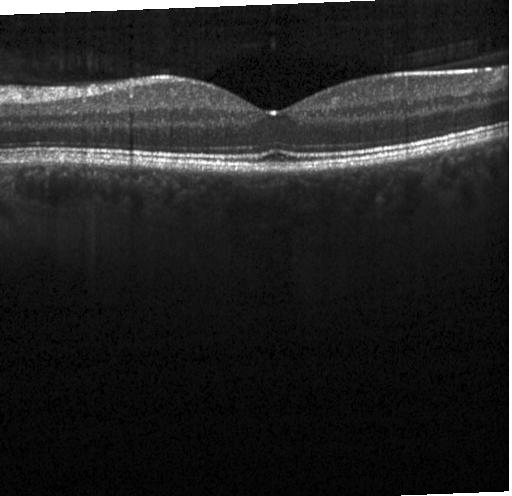
Spectral-domain OCT · Heidelberg Spectralis · retinal OCT B-scan.
The scan shows neither choroidal neovascularization, diabetic macular edema, nor drusen.